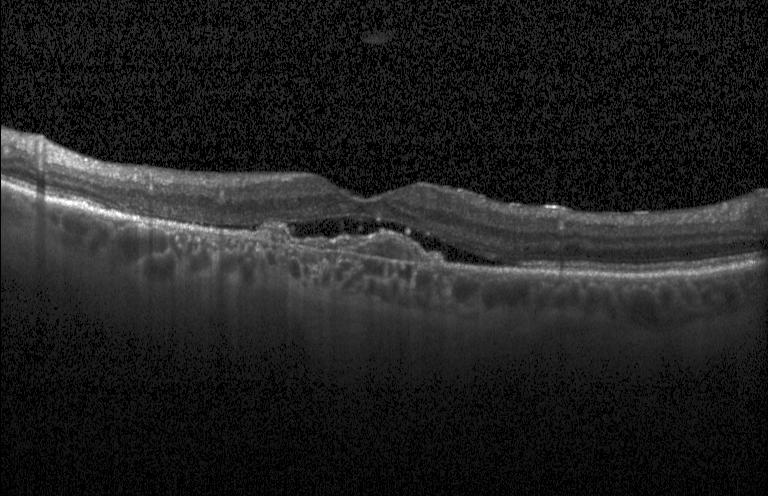

Spectral-domain OCT B-scan: a choroidal neovascular membrane.